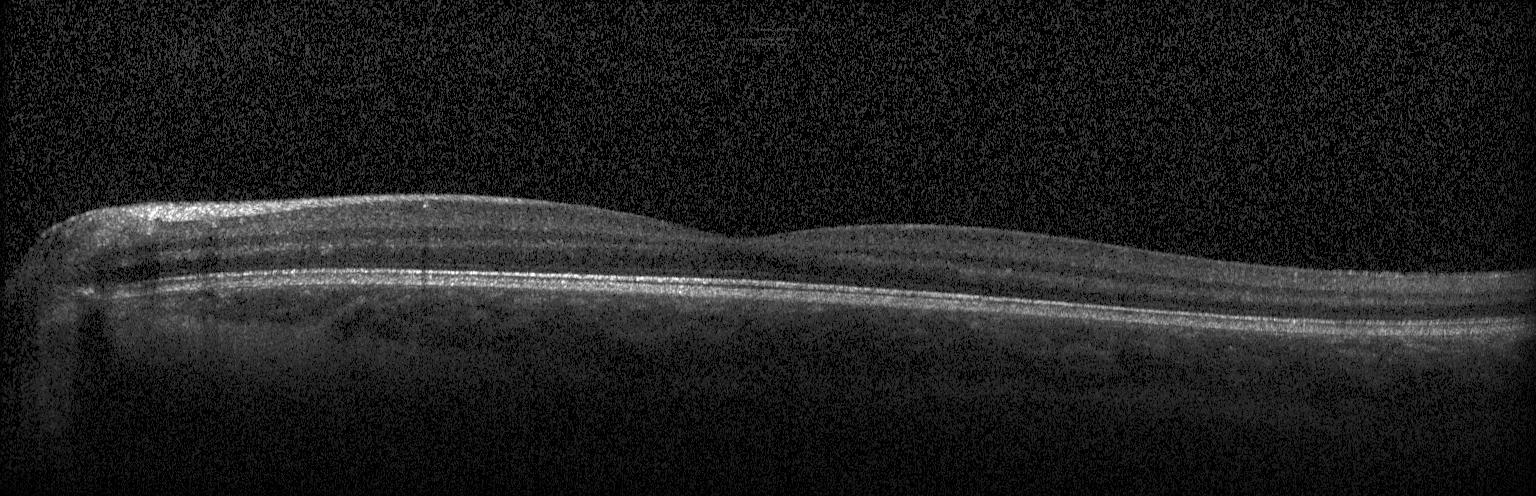
Centered on the fovea; Heidelberg Spectralis OCT system; OCT line scan
Impression: no choroidal neovascularization, no diabetic macular edema, and no drusen.